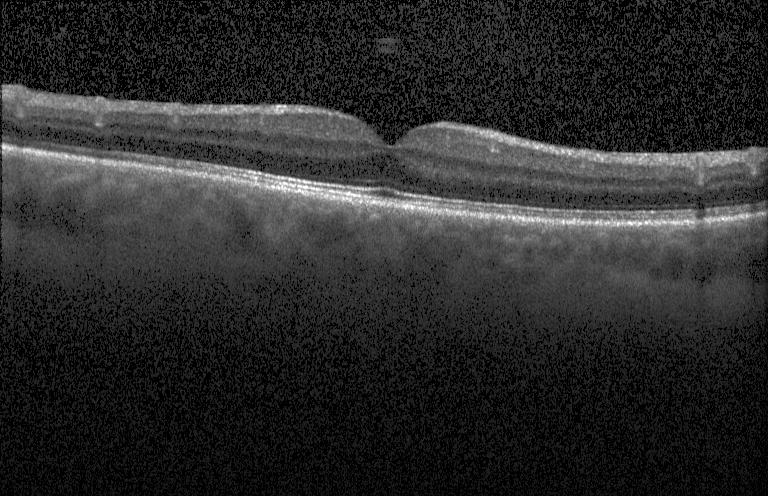
Horizontal scan through the fovea, spectral-domain OCT, retinal OCT cross-section — Finding: no choroidal neovascularization, no diabetic macular edema, and no drusen.